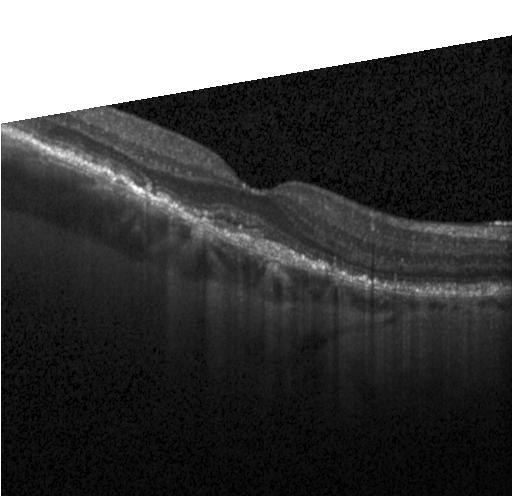
Acquired on a Heidelberg Spectralis, retinal OCT B-scan, SD-OCT, fovea-centered
Diagnosis: choroidal neovascularization (CNV).